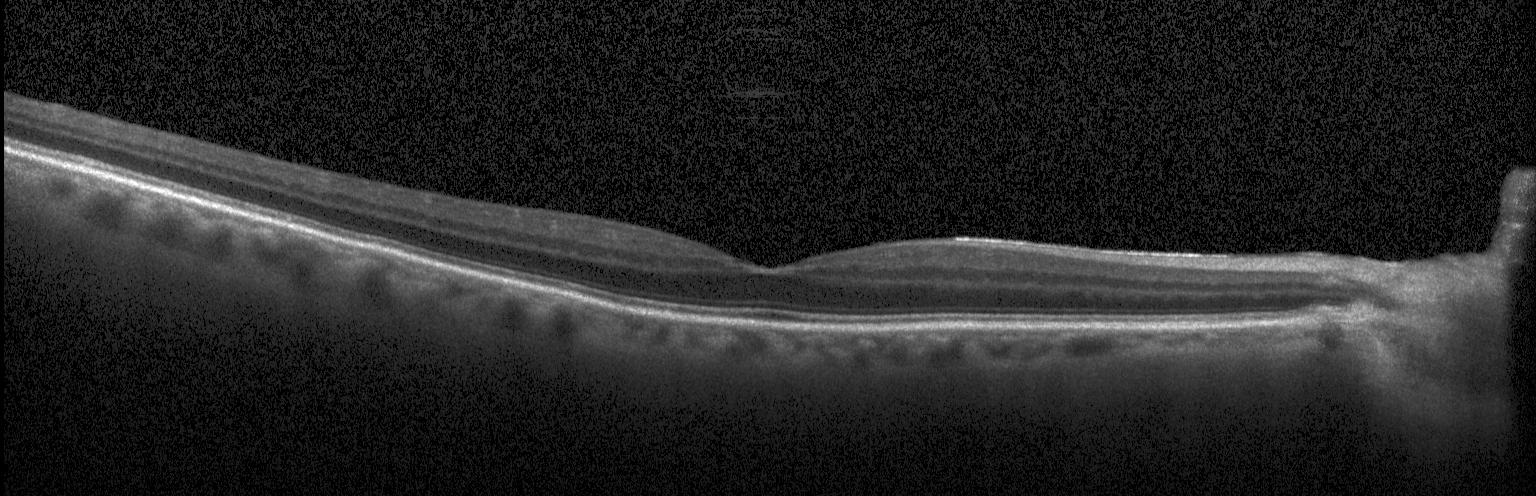

Dx: neither choroidal neovascularization, diabetic macular edema, nor drusen.